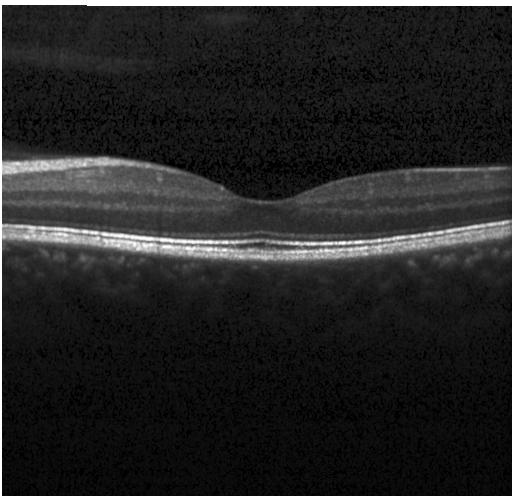 Retinal OCT B-scan · fovea-centered
Impression: no evidence of CNV, DME, or drusen.